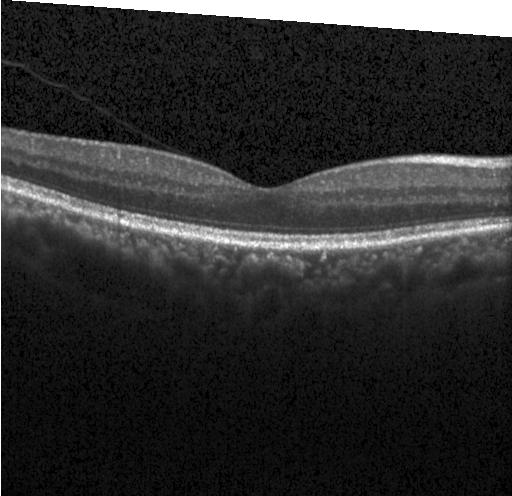
Retinal OCT cross-section
Macular OCT: neither CNV, DME, nor drusen.